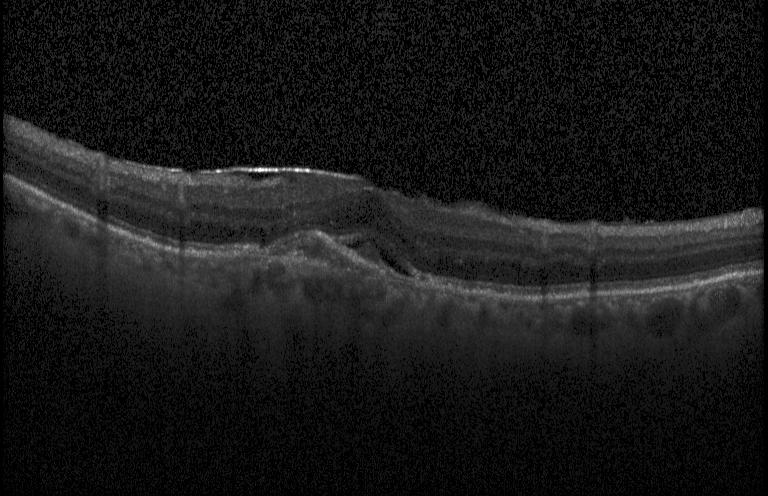
Spectral-domain OCT B-scan: choroidal neovascularization (CNV).